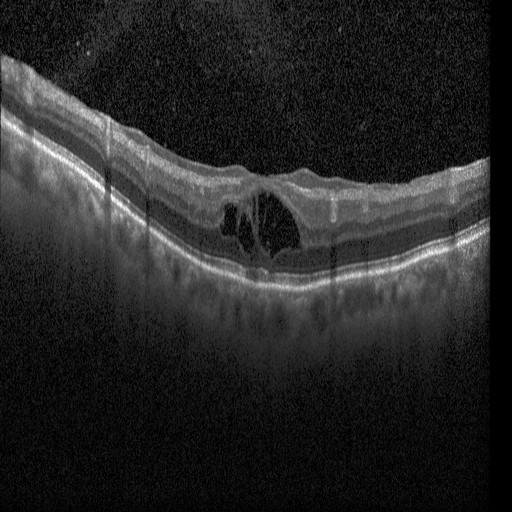 OCT scan showing diabetic macular edema (DME).